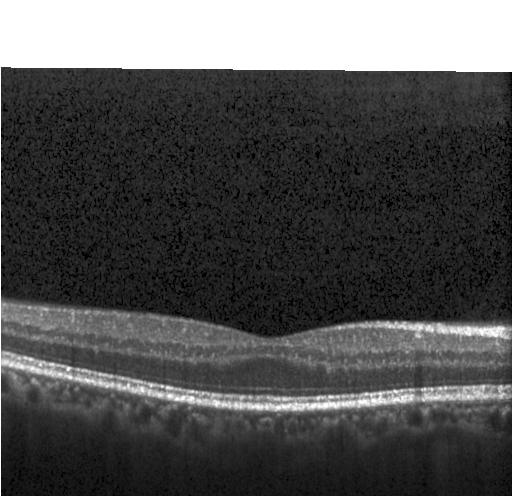 OCT B-scan. Finding: no choroidal neovascularization, diabetic macular edema, or drusen.